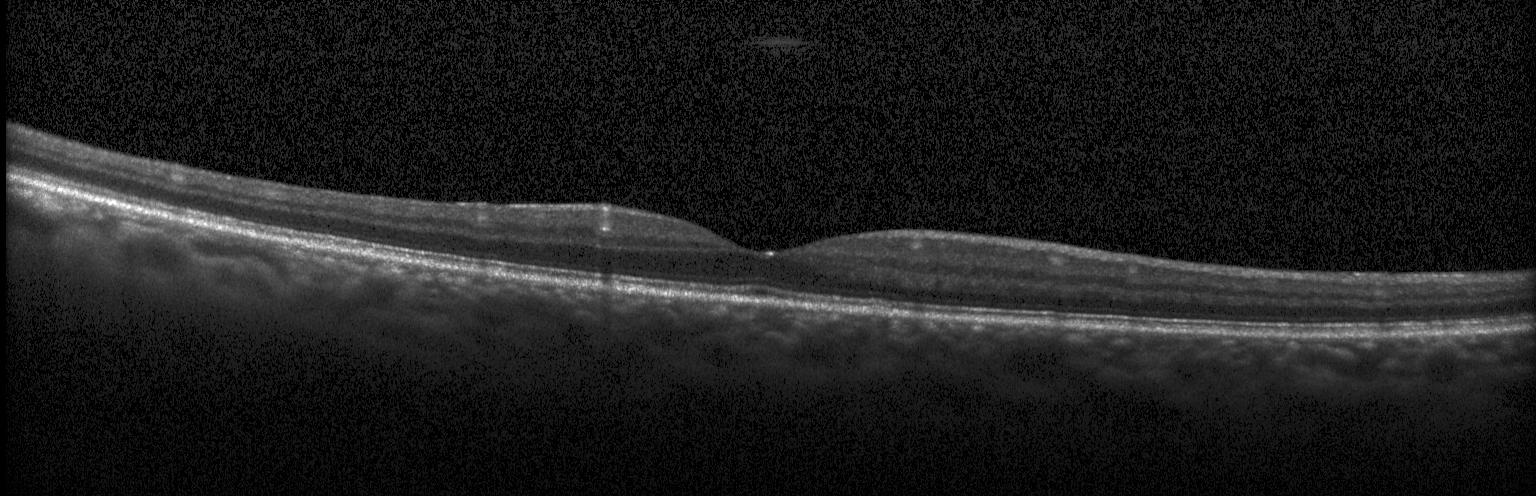
Spectral-domain OCT, OCT line scan, through the macula, Heidelberg Spectralis OCT system.
Impression: no choroidal neovascularization, diabetic macular edema, or drusen.